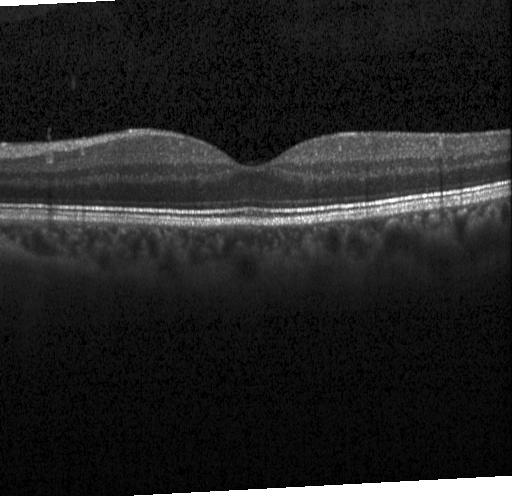 Retinal OCT B-scan. Spectral-domain OCT. Fovea-centered. Diagnosis: no evidence of choroidal neovascularization, diabetic macular edema, or drusen.